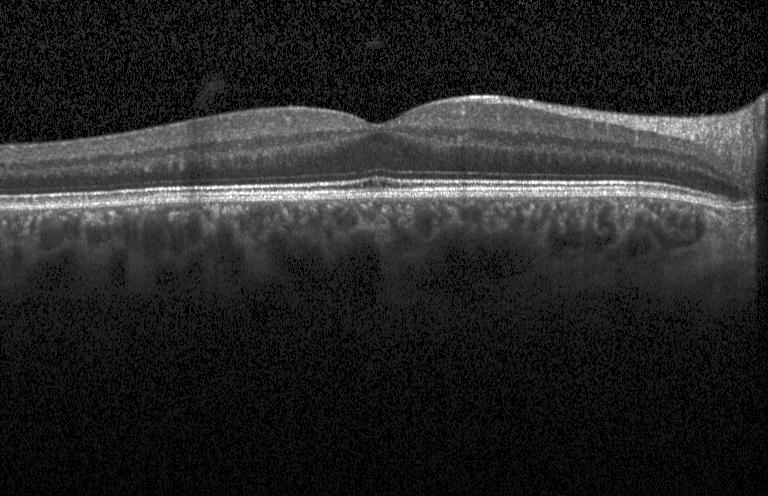 Heidelberg Spectralis; optical coherence tomography B-scan; spectral-domain OCT; centered on the fovea — Diagnosis: neither choroidal neovascularization, diabetic macular edema, nor drusen.